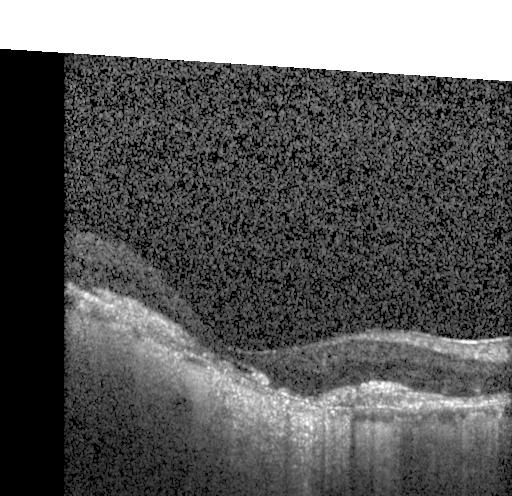

Optical coherence tomography scan. SD-OCT — Diagnosis: a choroidal neovascular membrane.